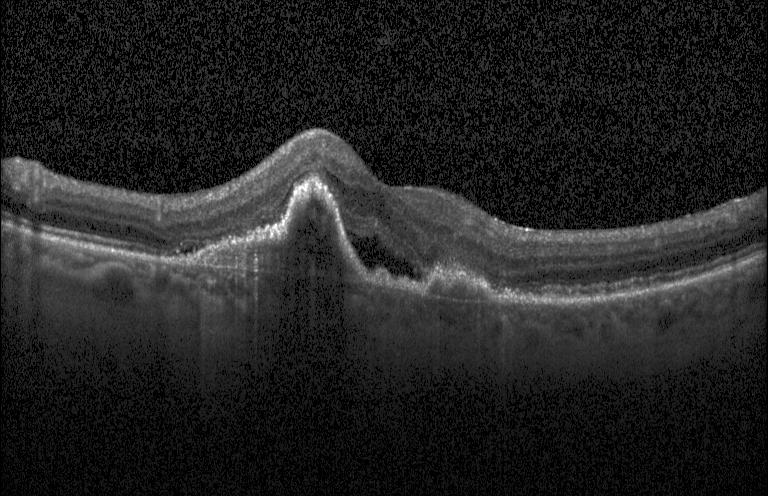

Assessment: CNV.